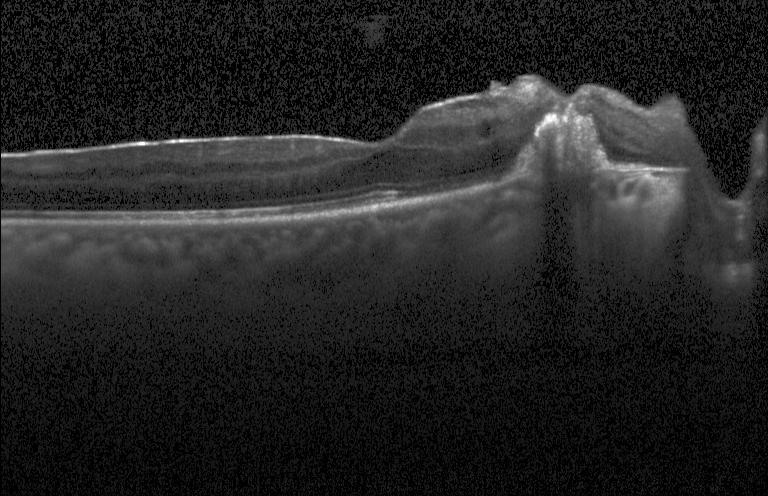 Optical coherence tomography scan; Heidelberg Spectralis OCT system; macular scan; SD-OCT.
Finding: a choroidal neovascular membrane.